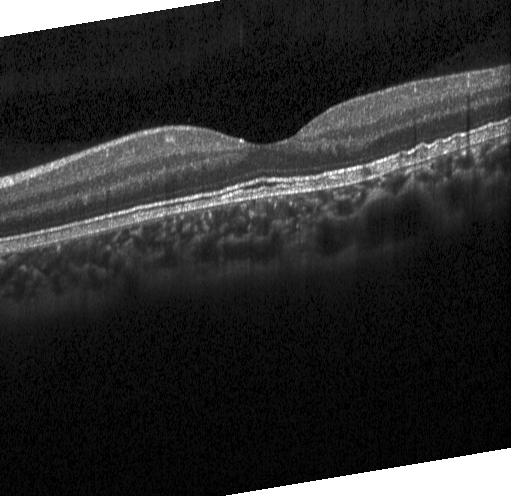

OCT B-scan. Instrument: Heidelberg Spectralis. SD-OCT — OCT finding: no choroidal neovascularization, diabetic macular edema, or drusen.